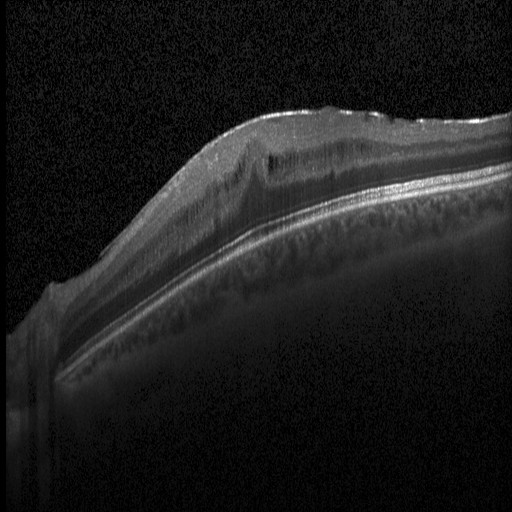

Heidelberg Spectralis; retinal OCT cross-section.
Finding: DME.